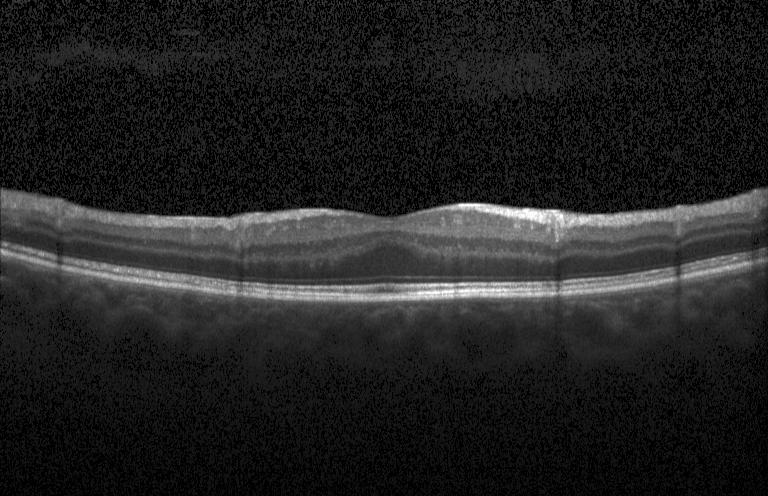
Finding: no CNV, DME, or drusen.